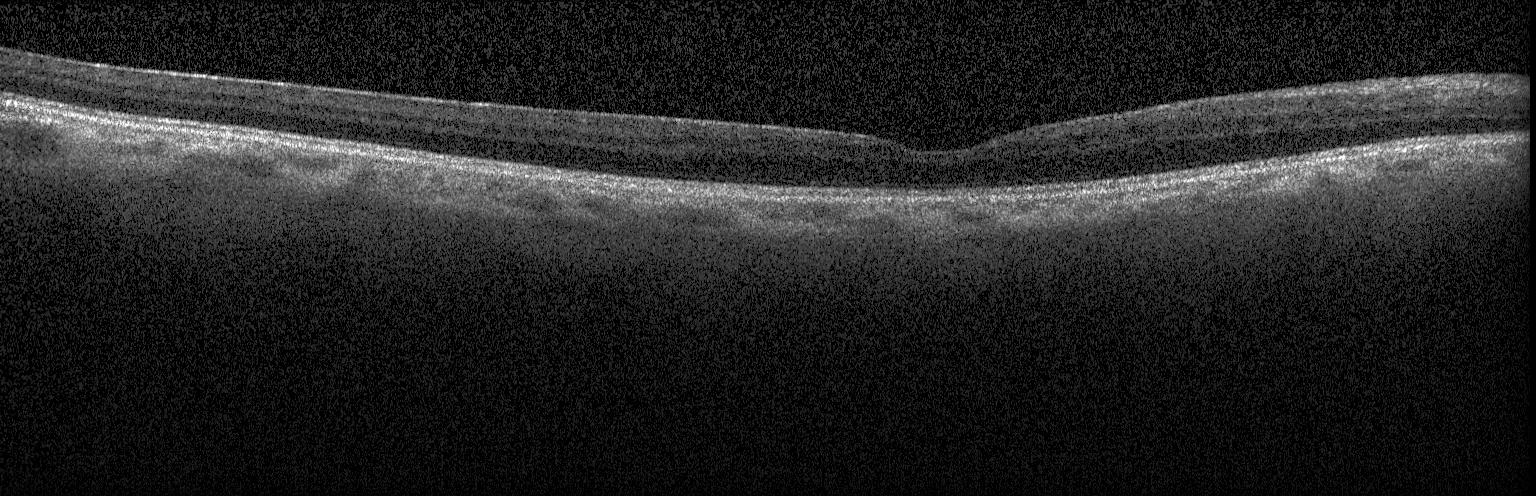
Optical coherence tomography B-scan · Heidelberg Spectralis OCT system
Finding: no CNV, DME, or drusen.